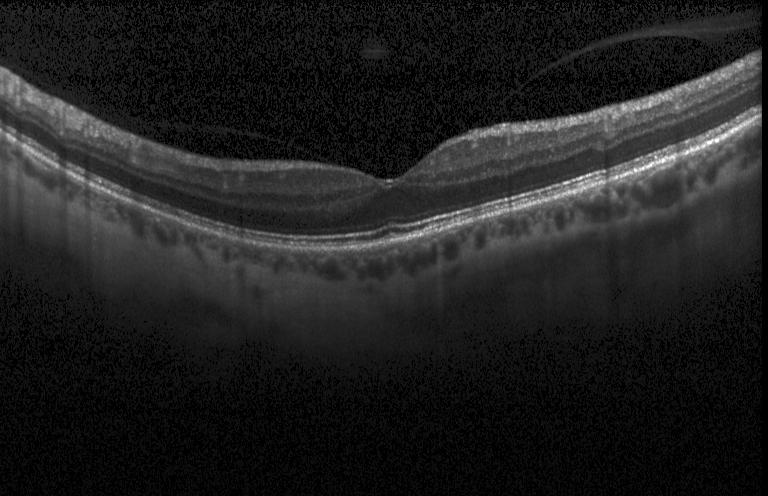 Spectral-domain OCT, horizontal scan through the fovea, instrument: Heidelberg Spectralis, optical coherence tomography scan — Impression: no evidence of CNV, DME, or drusen.